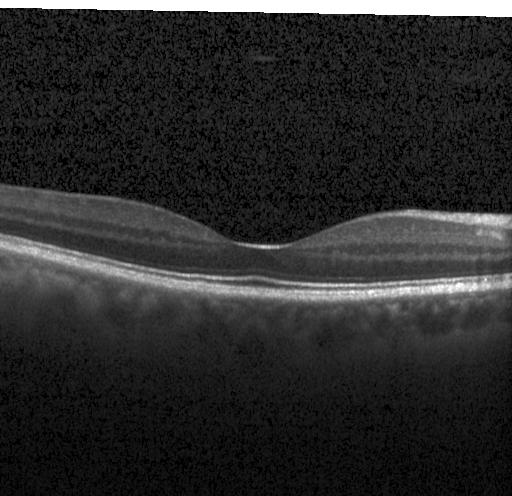 Macular OCT: neither CNV, DME, nor drusen.